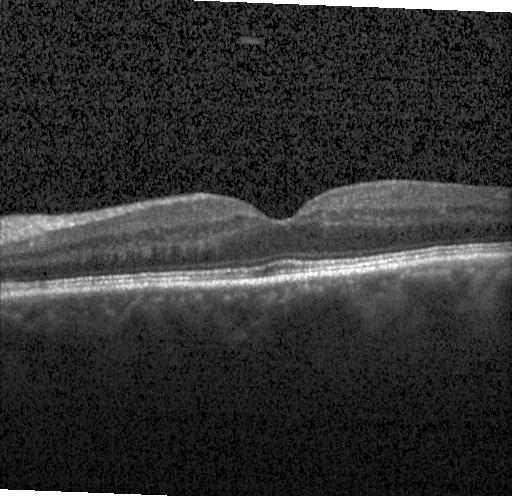

Instrument: Heidelberg Spectralis. OCT B-scan — Impression: no evidence of CNV, DME, or drusen.